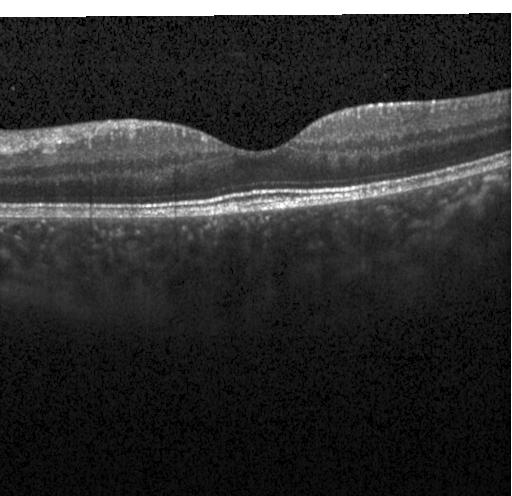 This B-scan demonstrates neither choroidal neovascularization, diabetic macular edema, nor drusen.